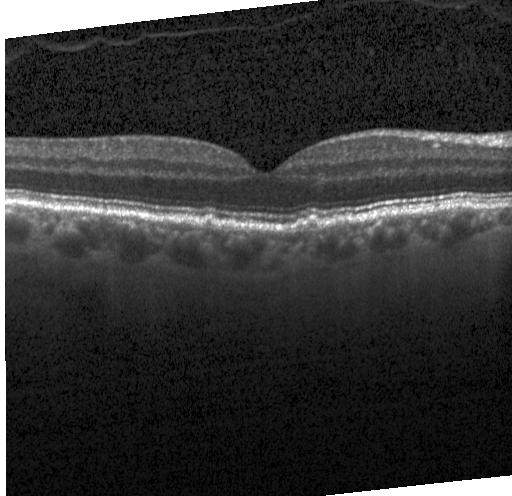

Fovea-centered · Heidelberg Spectralis · retinal OCT B-scan · spectral-domain optical coherence tomography — This B-scan demonstrates multiple drusen.